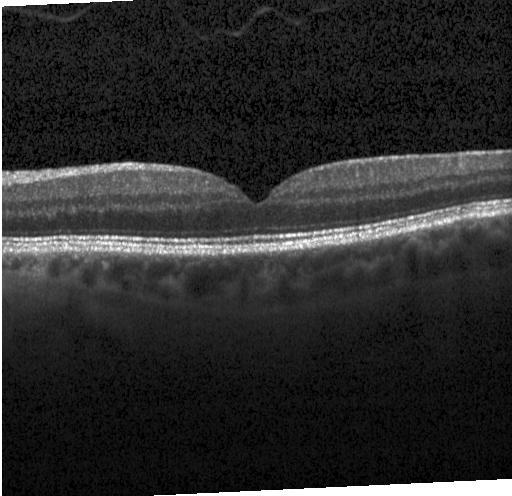
This B-scan demonstrates no choroidal neovascularization, no diabetic macular edema, and no drusen.